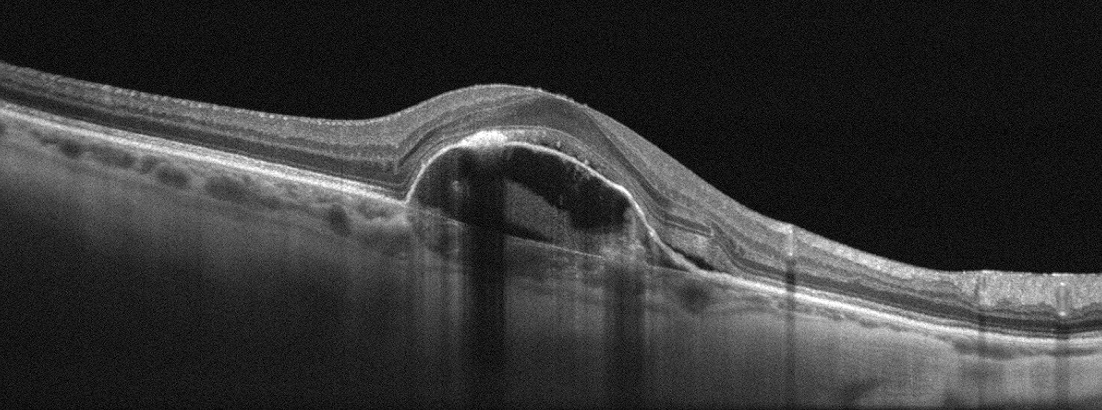 Macular OCT: age-related macular degeneration.